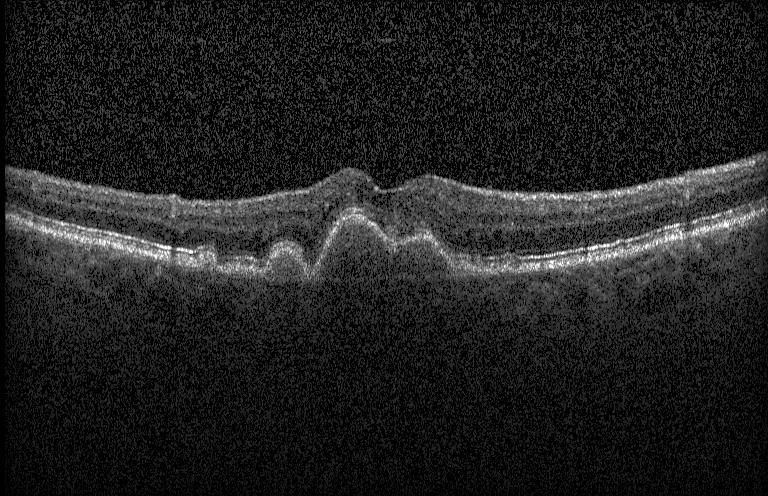
Spectral-domain optical coherence tomography, optical coherence tomography B-scan, horizontal scan through the fovea
This B-scan demonstrates choroidal neovascularization (CNV).